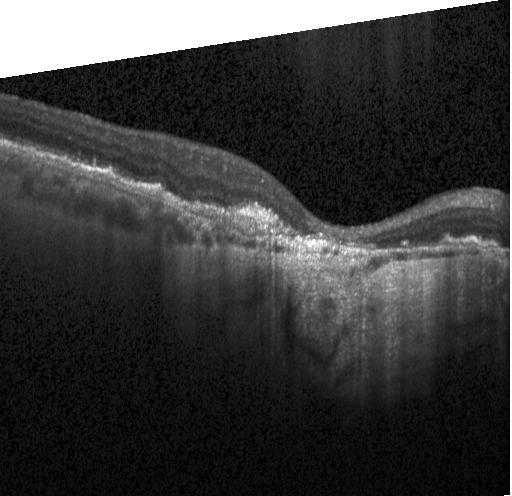
Macular OCT demonstrating choroidal neovascularization (CNV).